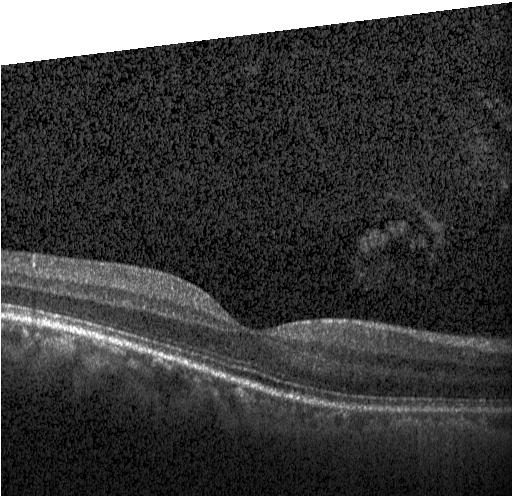

OCT B-scan. This B-scan demonstrates no evidence of CNV, DME, or drusen.